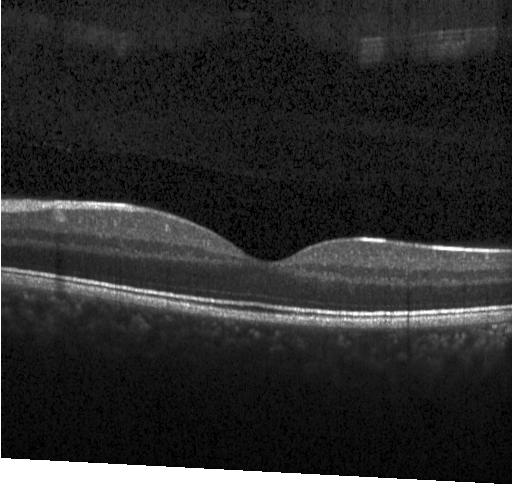

Retinal OCT cross-section — No evidence of choroidal neovascularization, diabetic macular edema, or drusen.